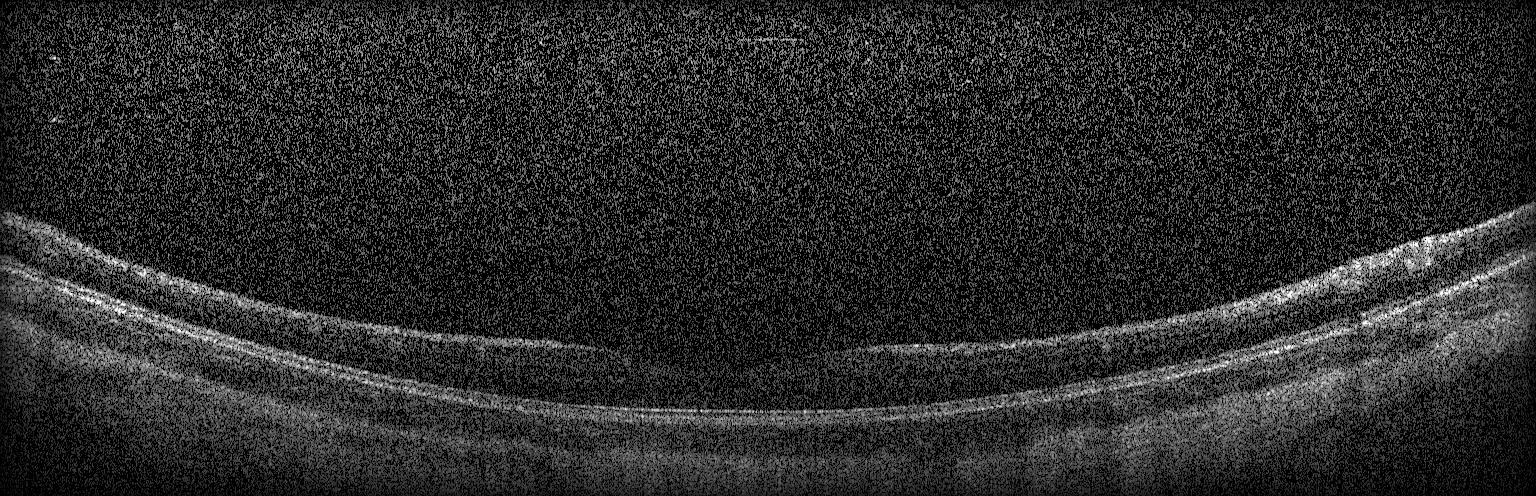 OCT line scan. Spectral-domain optical coherence tomography
This B-scan demonstrates no evidence of CNV, DME, or drusen.